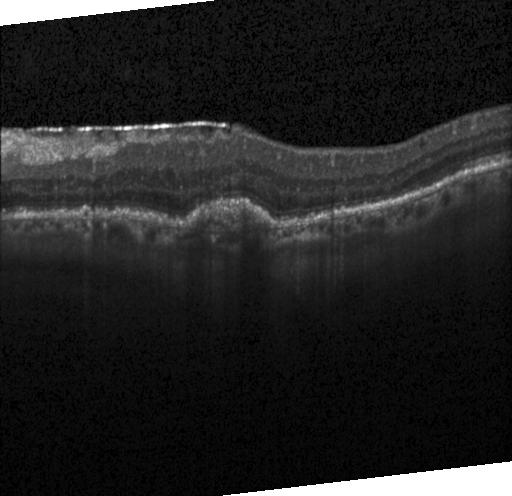
Spectral-domain OCT · Heidelberg Spectralis OCT system · through the macula · OCT B-scan
OCT finding: a choroidal neovascular membrane.